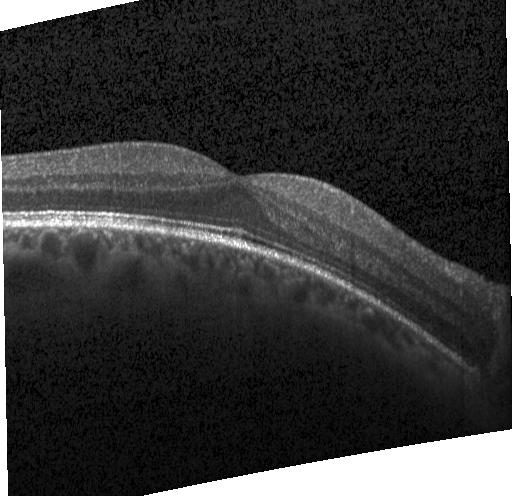
Optical coherence tomography B-scan.
Dx: no choroidal neovascularization, diabetic macular edema, or drusen.